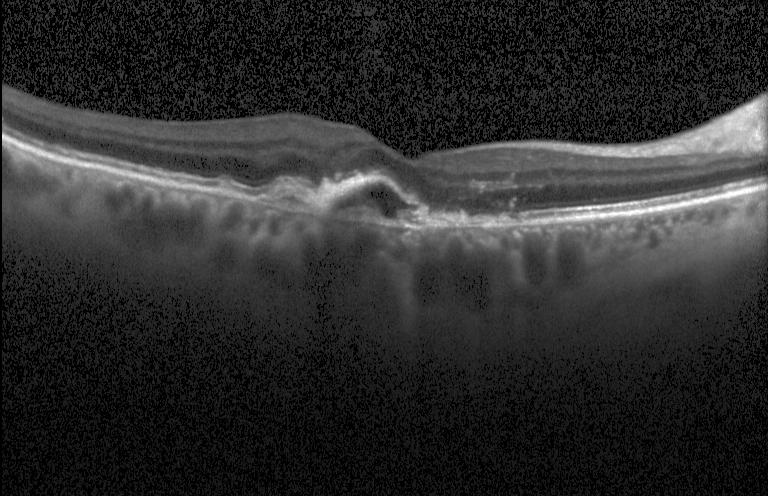

Spectral-domain OCT. Retinal OCT B-scan. Dx: a choroidal neovascular membrane.